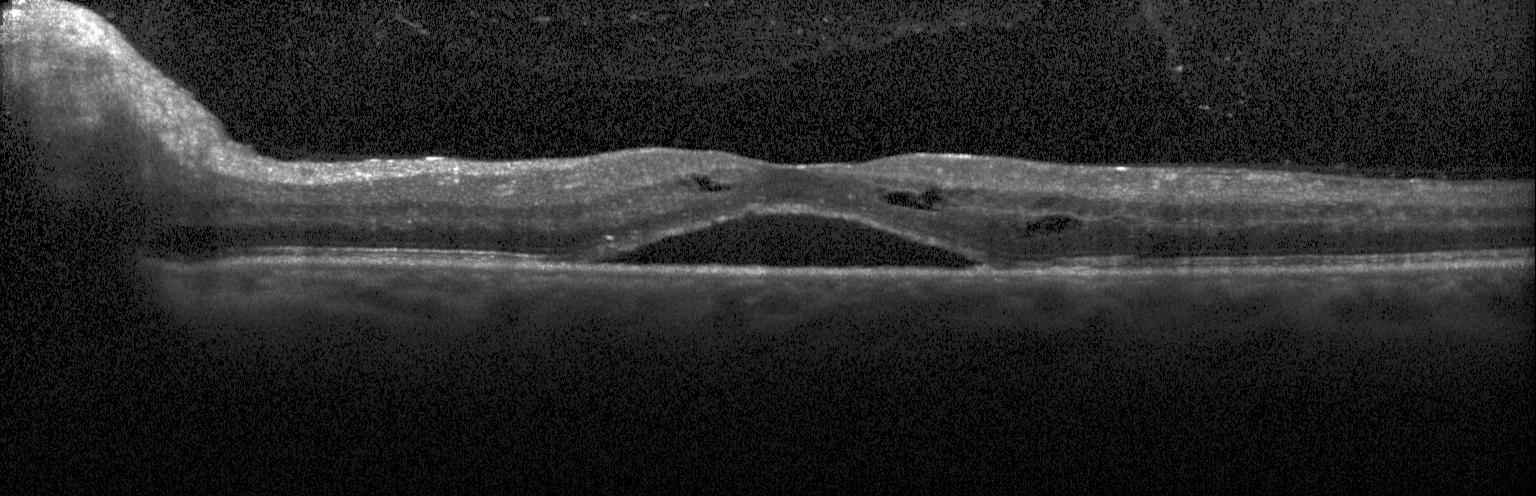 OCT B-scan · spectral-domain optical coherence tomography. The scan shows diabetic macular edema.